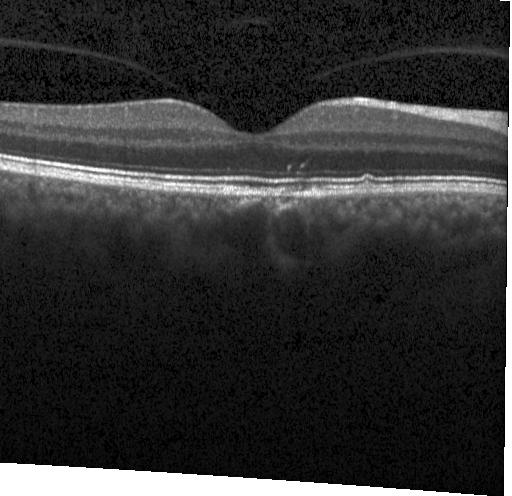 Instrument: Heidelberg Spectralis. Optical coherence tomography B-scan — Assessment: drusen.